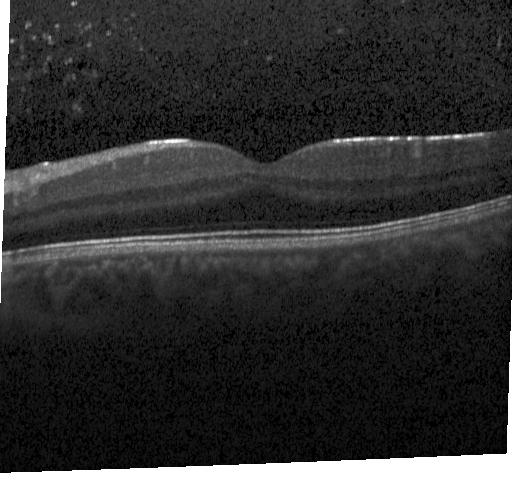
OCT line scan.
No CNV, DME, or drusen.